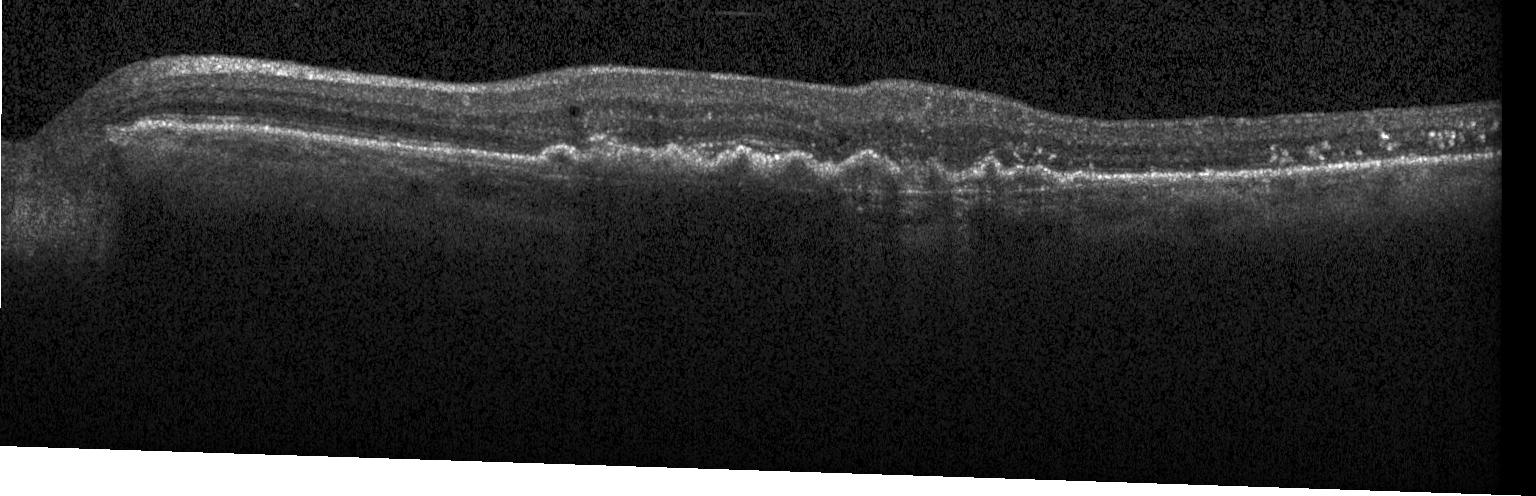

Spectral-domain OCT B-scan: a choroidal neovascular membrane.